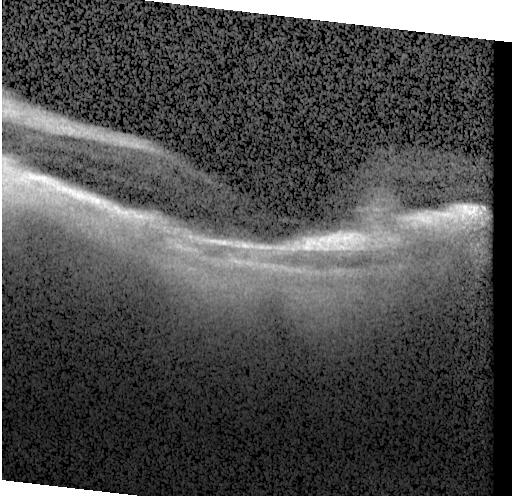
Spectral-domain OCT B-scan: choroidal neovascularization (CNV).